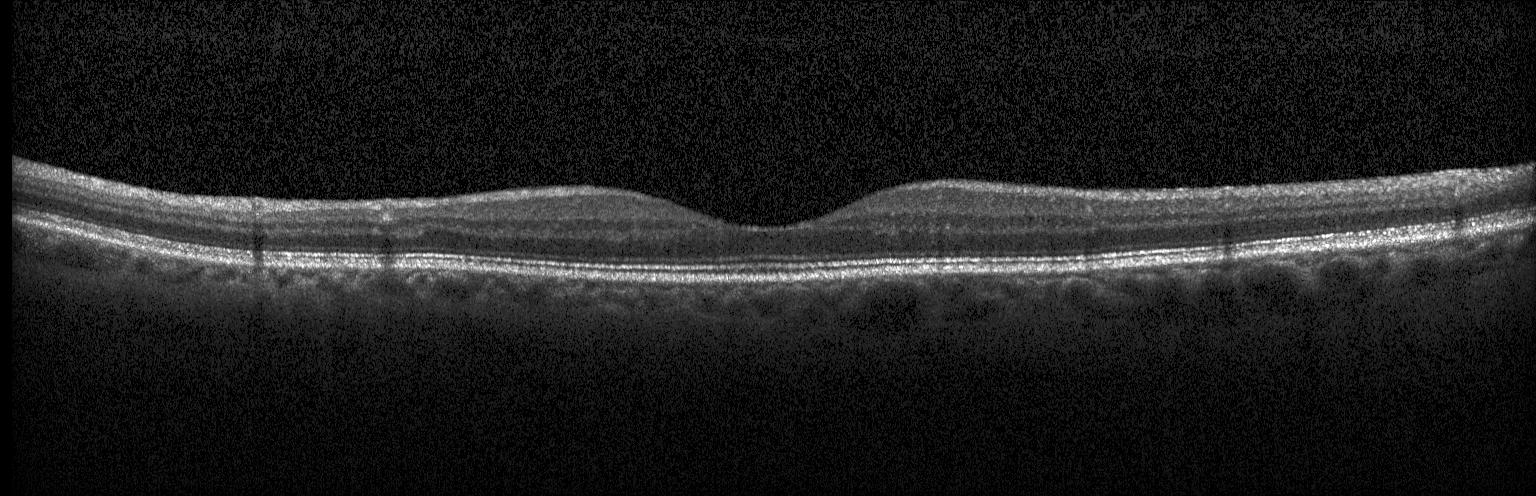
OCT line scan, fovea-centered. Assessment: no choroidal neovascularization, diabetic macular edema, or drusen.